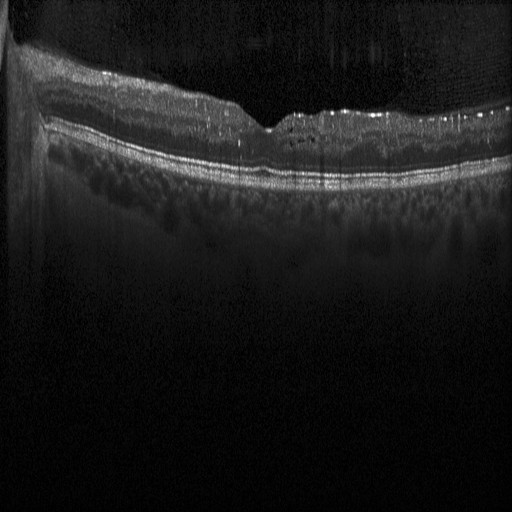
Retinal OCT cross-section showing DME.